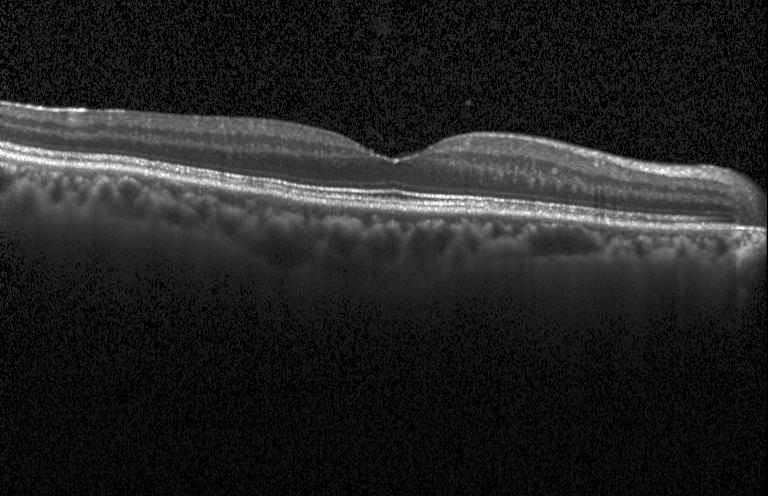
OCT line scan.
Assessment: no evidence of choroidal neovascularization, diabetic macular edema, or drusen.